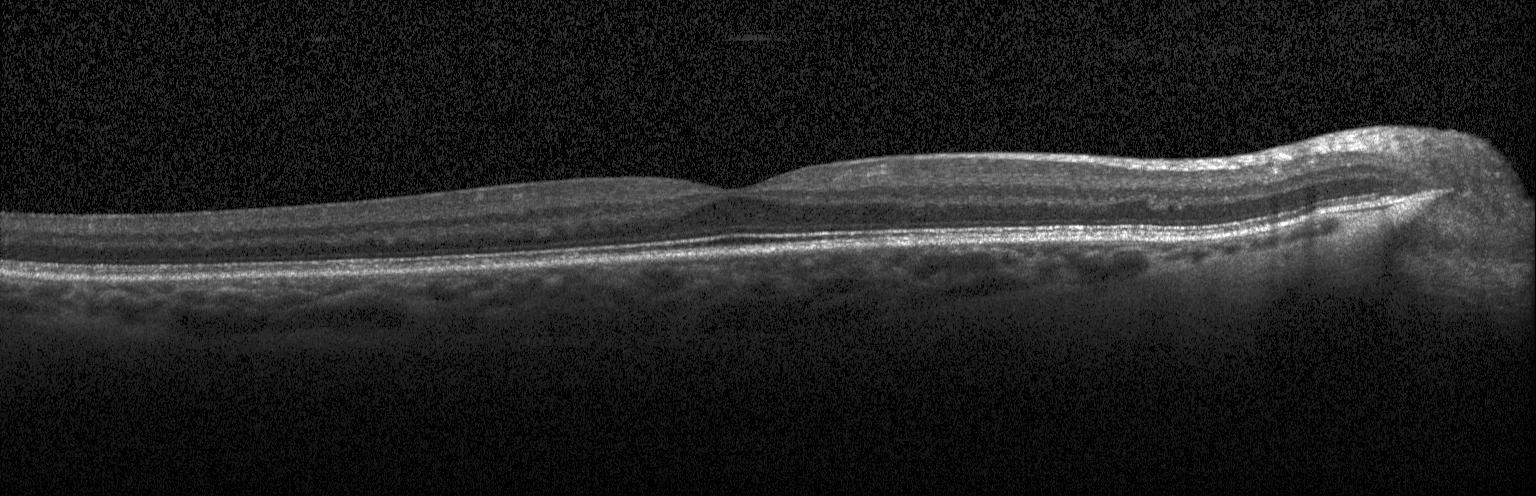
Macular scan · retinal OCT cross-section
Impression: no choroidal neovascularization, no diabetic macular edema, and no drusen.